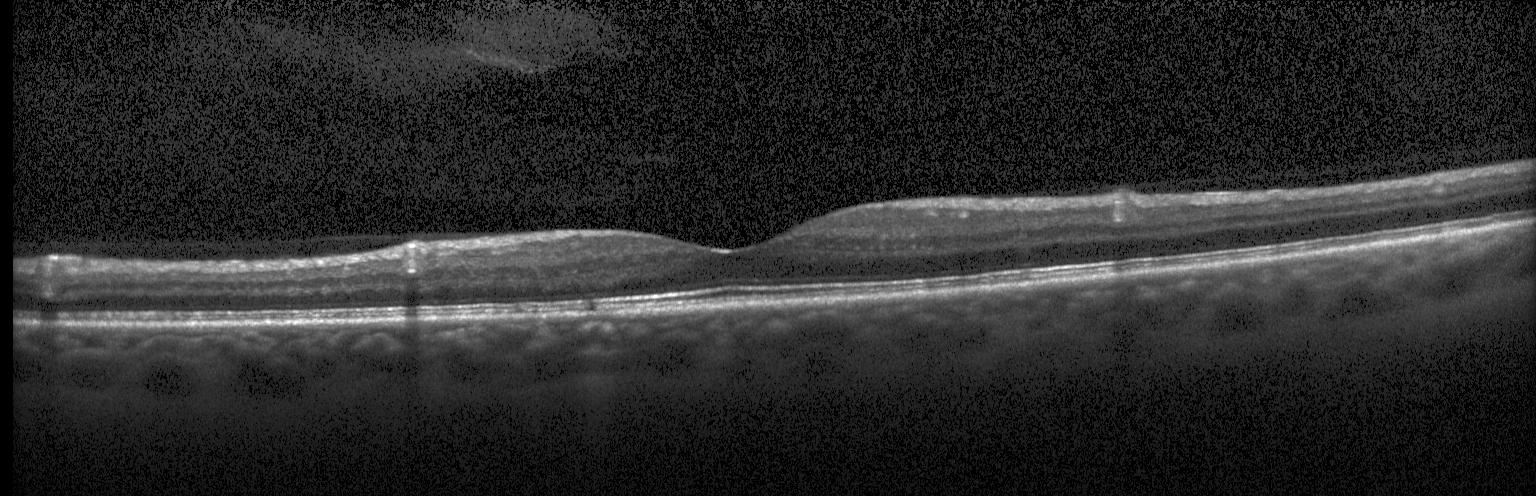
Dx: no choroidal neovascularization, no diabetic macular edema, and no drusen.